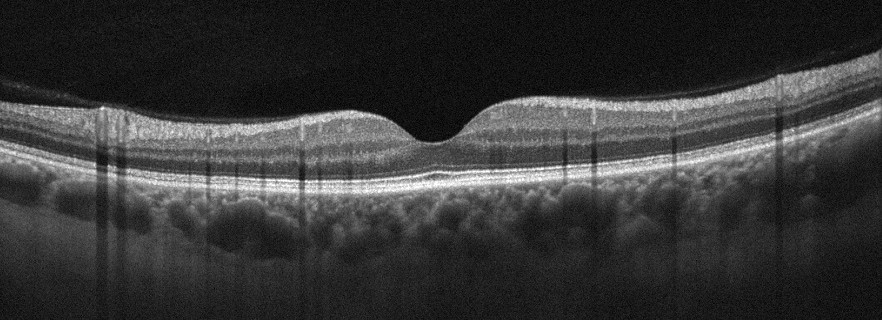
Instrument: Optovue Avanti RTVue XR · through the macula · OCT B-scan.
Finding: absence of AMD, DME, ERM, RAO, RVO, and vitreomacular interface disease.